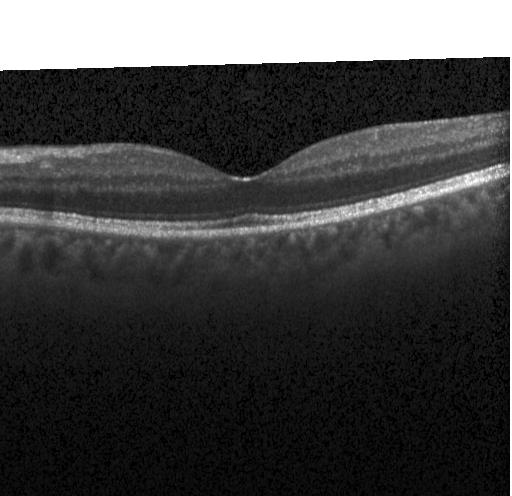
OCT line scan, acquired on a Heidelberg Spectralis, centered on the fovea, spectral-domain OCT. No evidence of CNV, DME, or drusen.